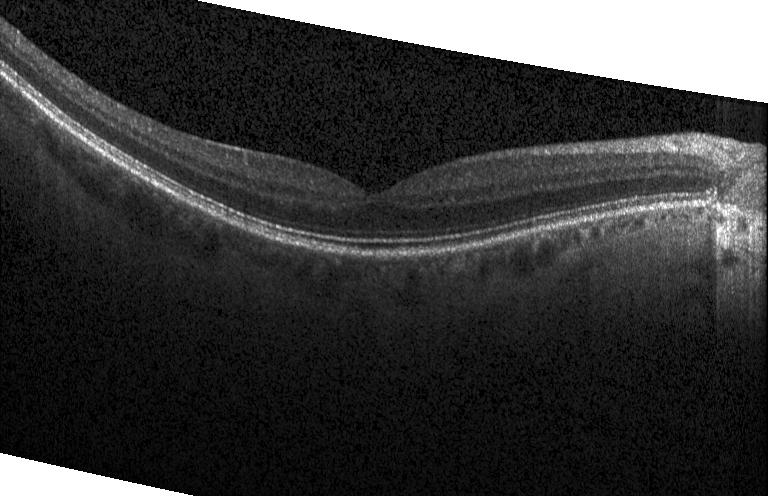
OCT B-scan · macular scan.
Finding: no evidence of choroidal neovascularization, diabetic macular edema, or drusen.